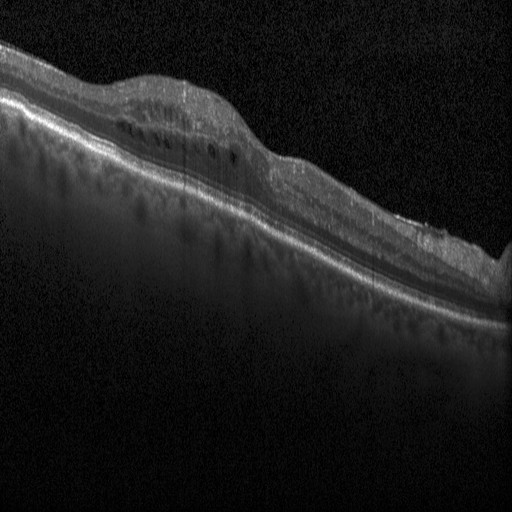
Spectral-domain OCT B-scan: DME.